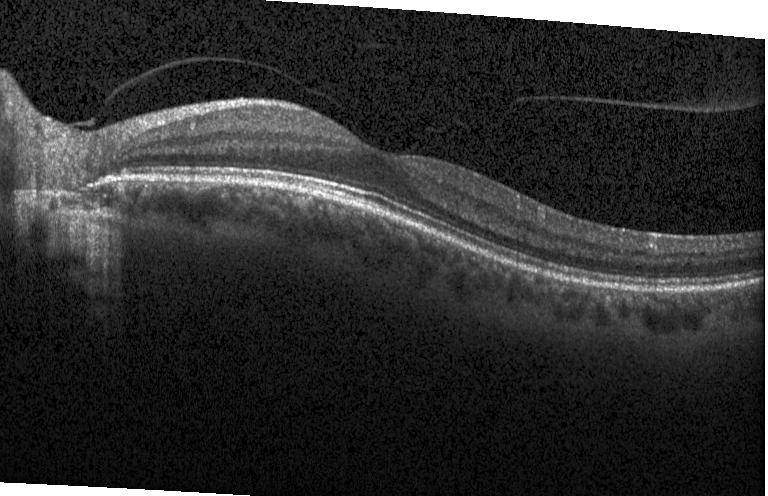
OCT finding: neither choroidal neovascularization, diabetic macular edema, nor drusen.